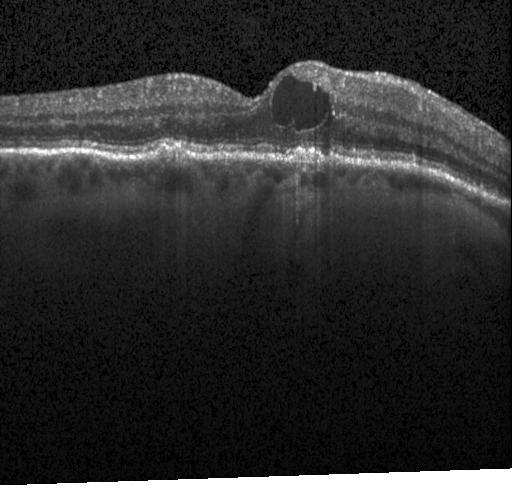
Retinal OCT B-scan — Diagnosis: choroidal neovascularization.